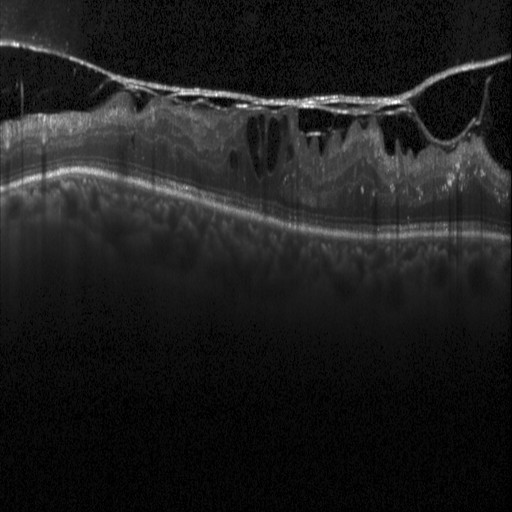 Retinal OCT cross-section.
This B-scan demonstrates diabetic macular edema (DME).